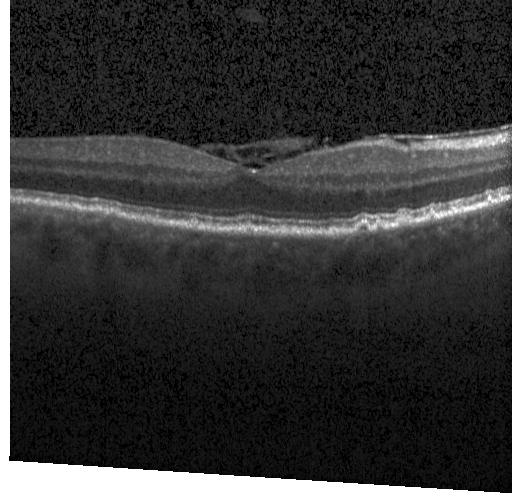

OCT B-scan. Diagnosis: sub-RPE drusenoid deposits.